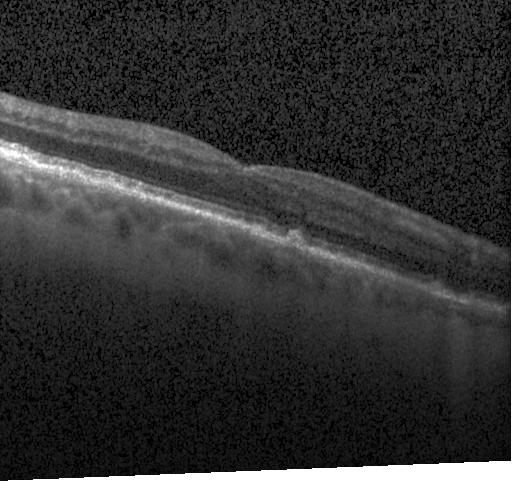 Finding: sub-RPE drusenoid deposits.